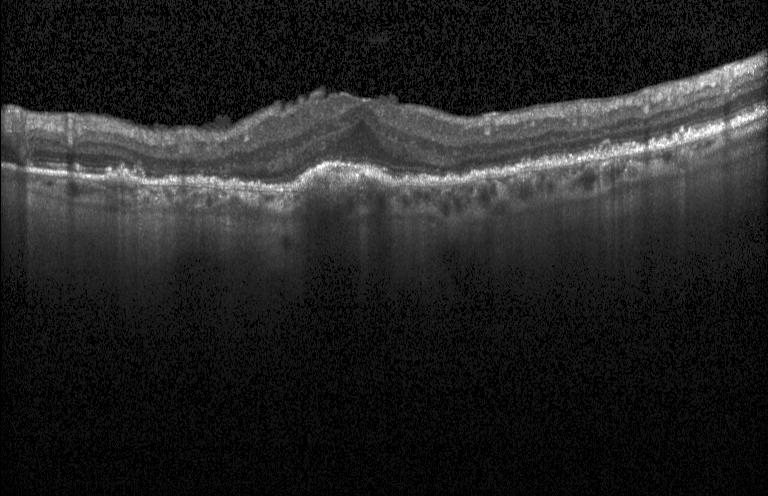
Spectral-domain optical coherence tomography · OCT line scan. OCT finding: a choroidal neovascular membrane.